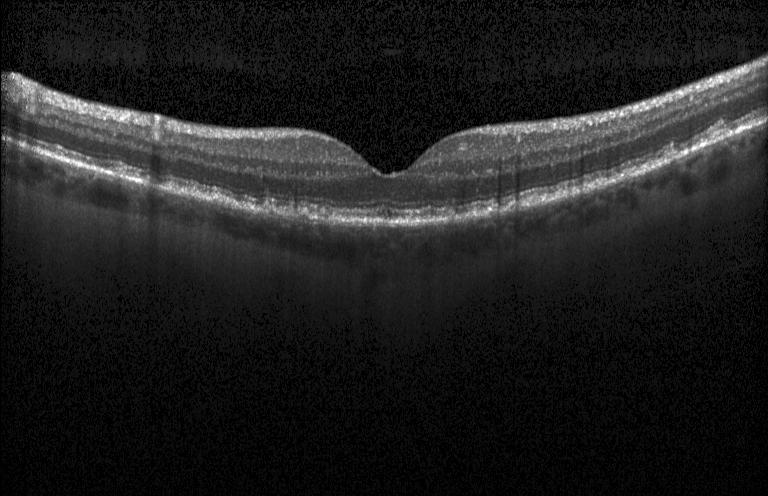

OCT line scan.
Diagnosis: sub-RPE drusenoid deposits.